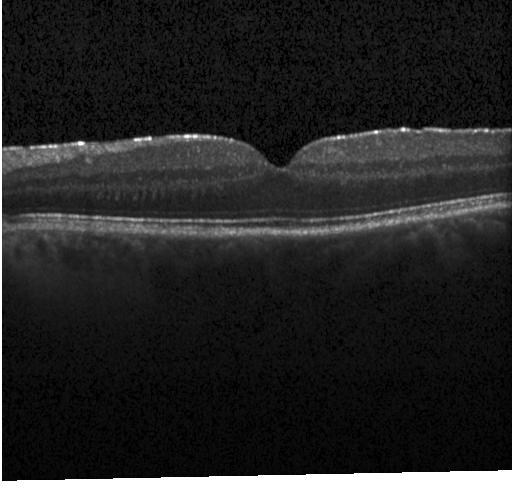 Macular scan, Heidelberg Spectralis OCT system, optical coherence tomography scan
OCT finding: no evidence of CNV, DME, or drusen.